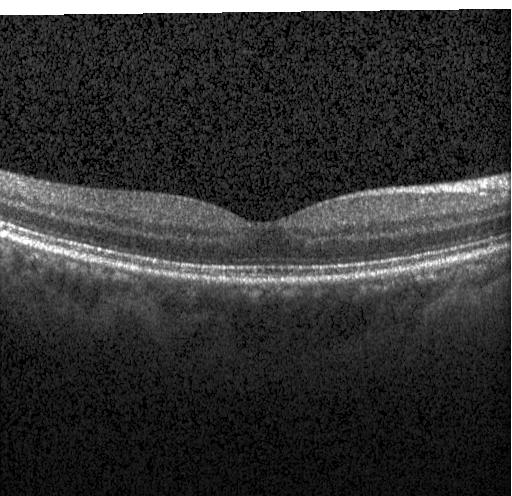

Retinal OCT B-scan
Finding: no choroidal neovascularization, diabetic macular edema, or drusen.